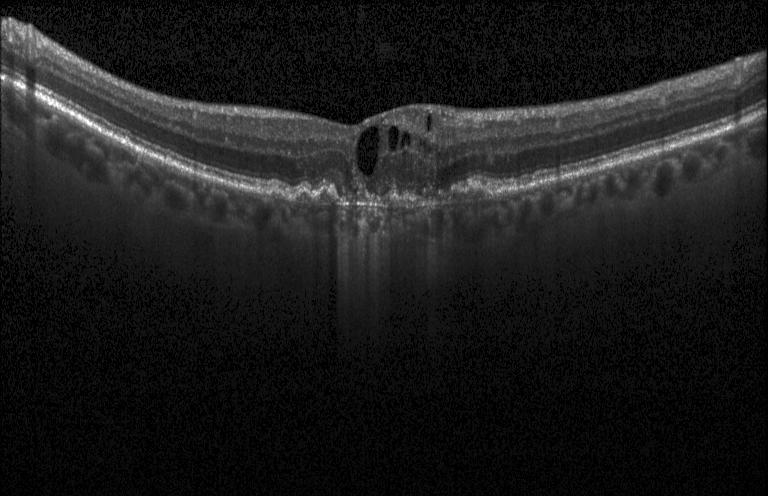 OCT scan showing a choroidal neovascular membrane.